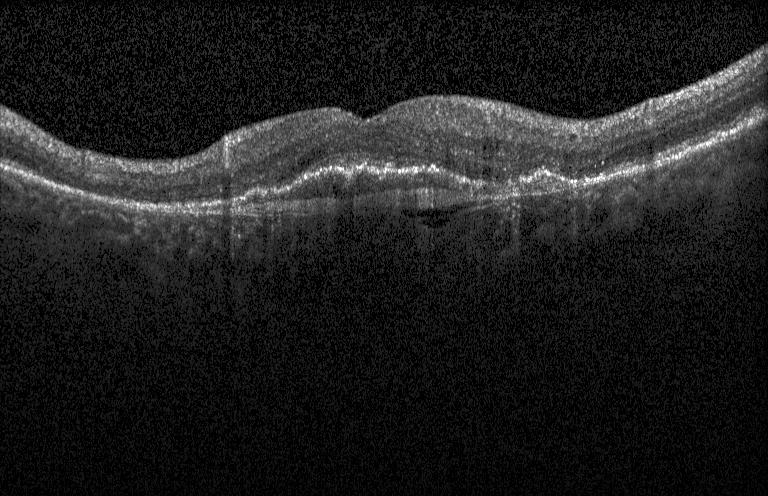
CNV.